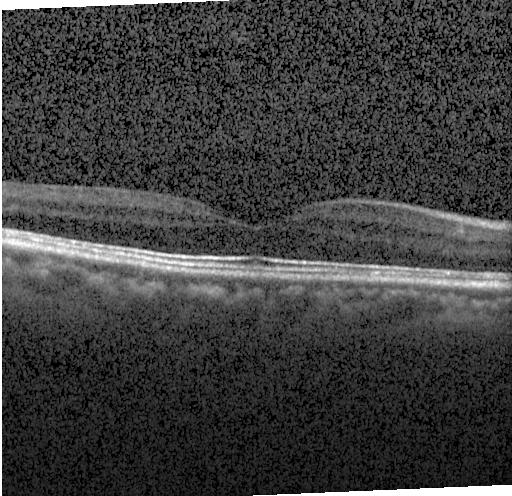 Fovea-centered; SD-OCT; retinal OCT cross-section
Dx: neither choroidal neovascularization, diabetic macular edema, nor drusen.